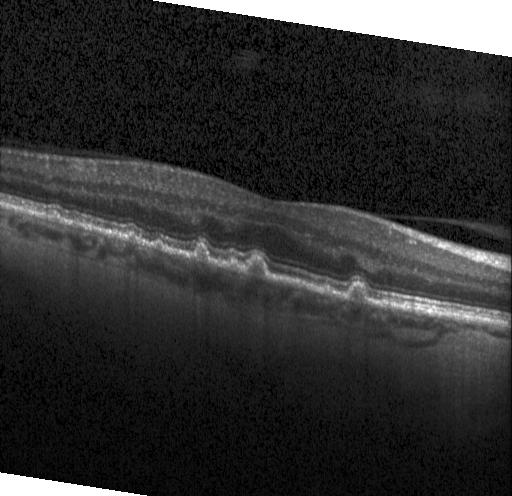

Centered on the fovea · OCT line scan. This B-scan demonstrates drusen.